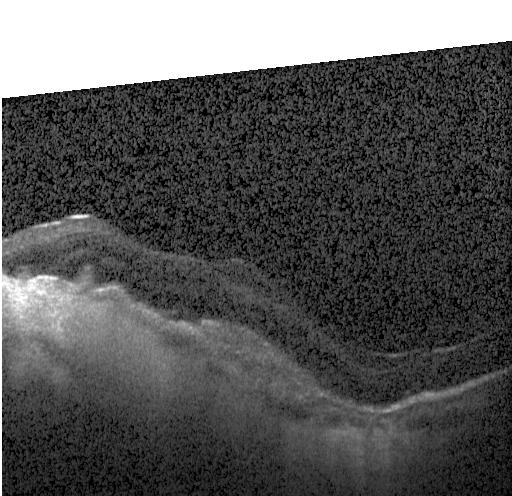 Finding: a choroidal neovascular membrane.